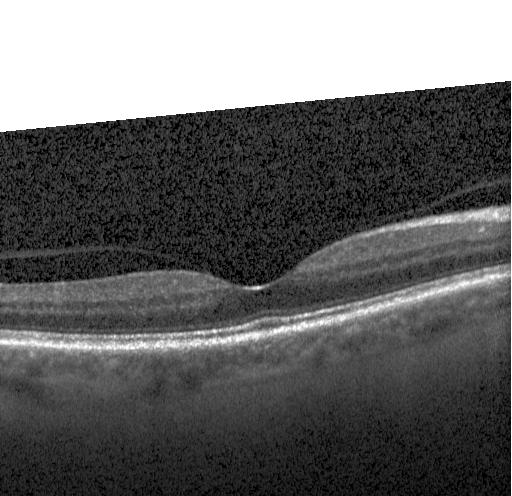 Fovea-centered, acquired on a Heidelberg Spectralis, spectral-domain optical coherence tomography, retinal OCT B-scan. Impression: no evidence of CNV, DME, or drusen.